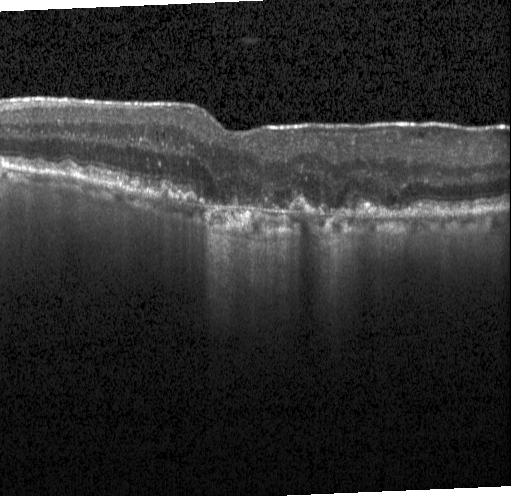

Optical coherence tomography scan
Dx: a choroidal neovascular membrane.